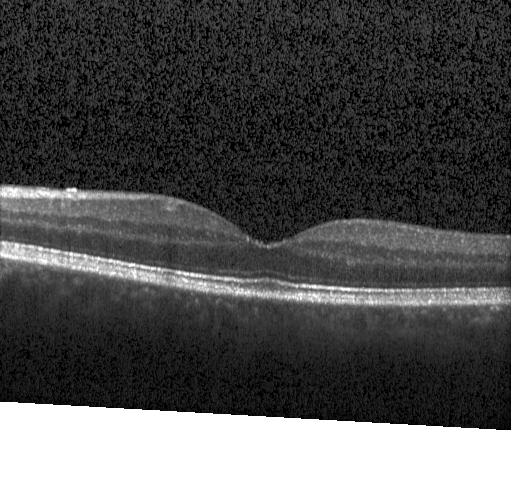 Spectral-domain optical coherence tomography, Heidelberg Spectralis OCT system, OCT line scan. OCT finding: no evidence of choroidal neovascularization, diabetic macular edema, or drusen.